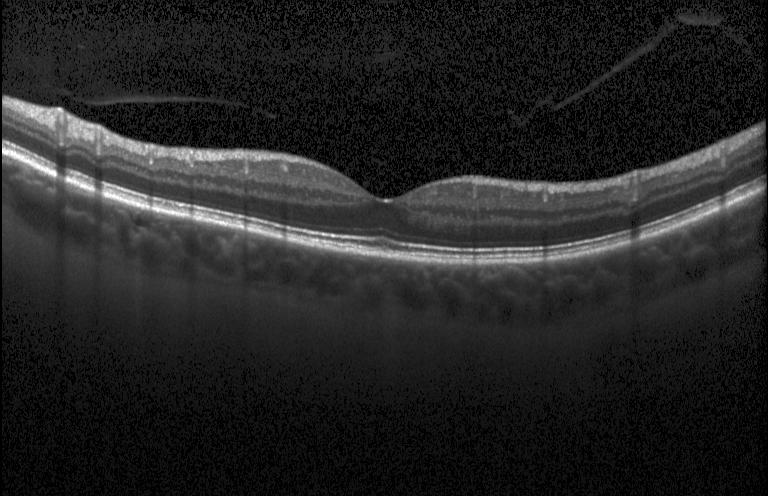

Optical coherence tomography B-scan — No evidence of CNV, DME, or drusen.